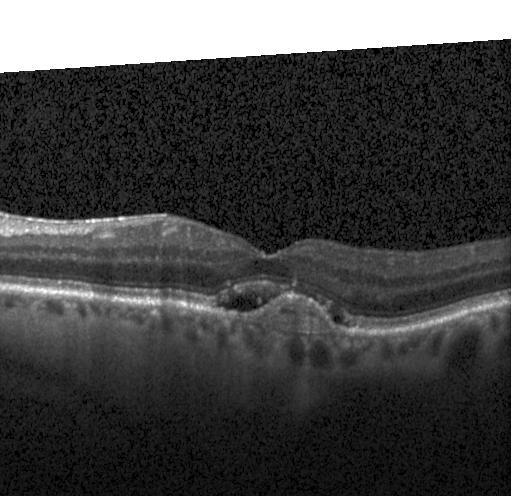 Through the macula; spectral-domain optical coherence tomography; OCT line scan. Impression: choroidal neovascularization.